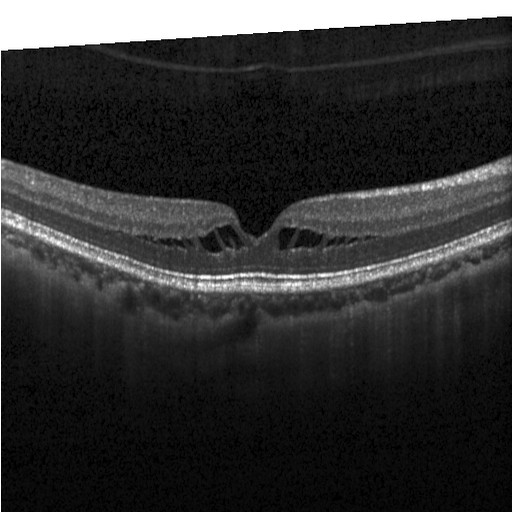
Optical coherence tomography B-scan — Impression: diabetic macular edema.